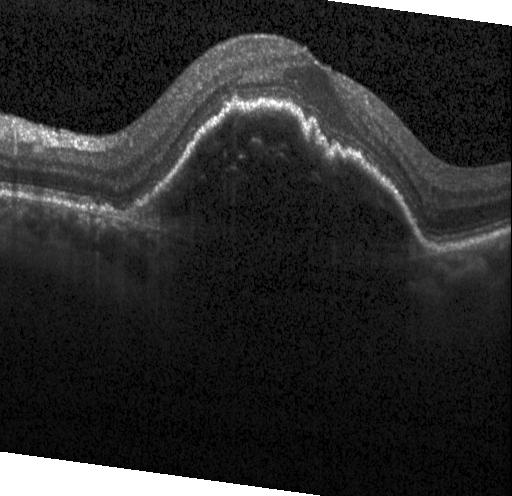 Through the macula. OCT B-scan. SD-OCT. Instrument: Heidelberg Spectralis.
This B-scan demonstrates a choroidal neovascular membrane.